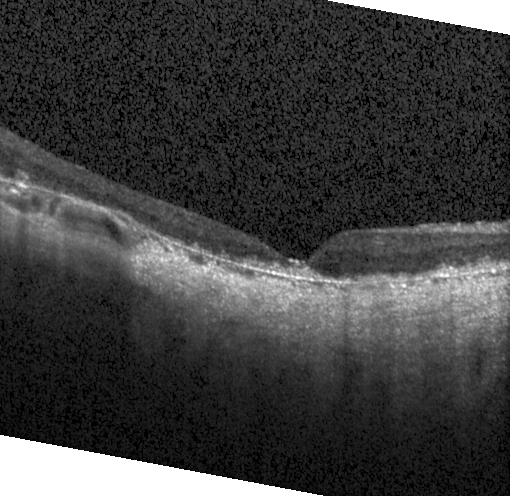

SD-OCT. Optical coherence tomography scan — The scan shows a choroidal neovascular membrane.